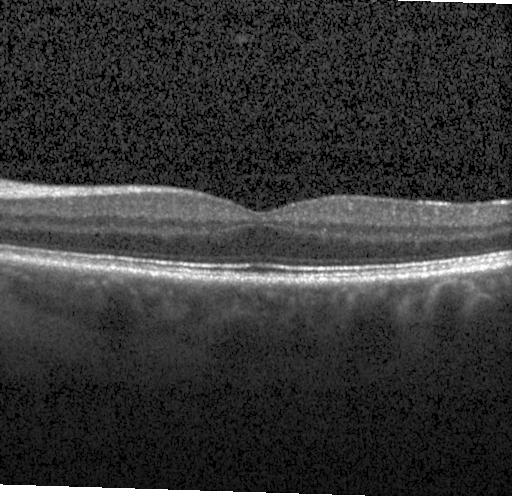

OCT finding: no CNV, DME, or drusen.